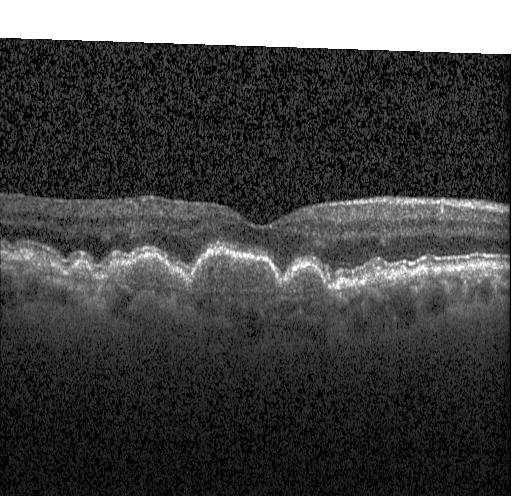
Optical coherence tomography B-scan
Sub-RPE drusenoid deposits.